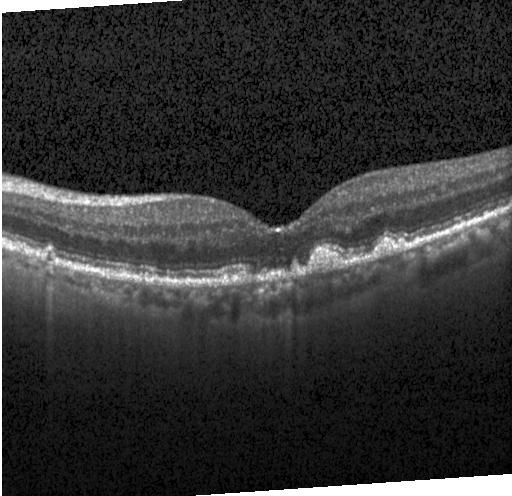

Heidelberg Spectralis. Spectral-domain optical coherence tomography. Horizontal scan through the fovea. Retinal OCT B-scan
Multiple drusen.